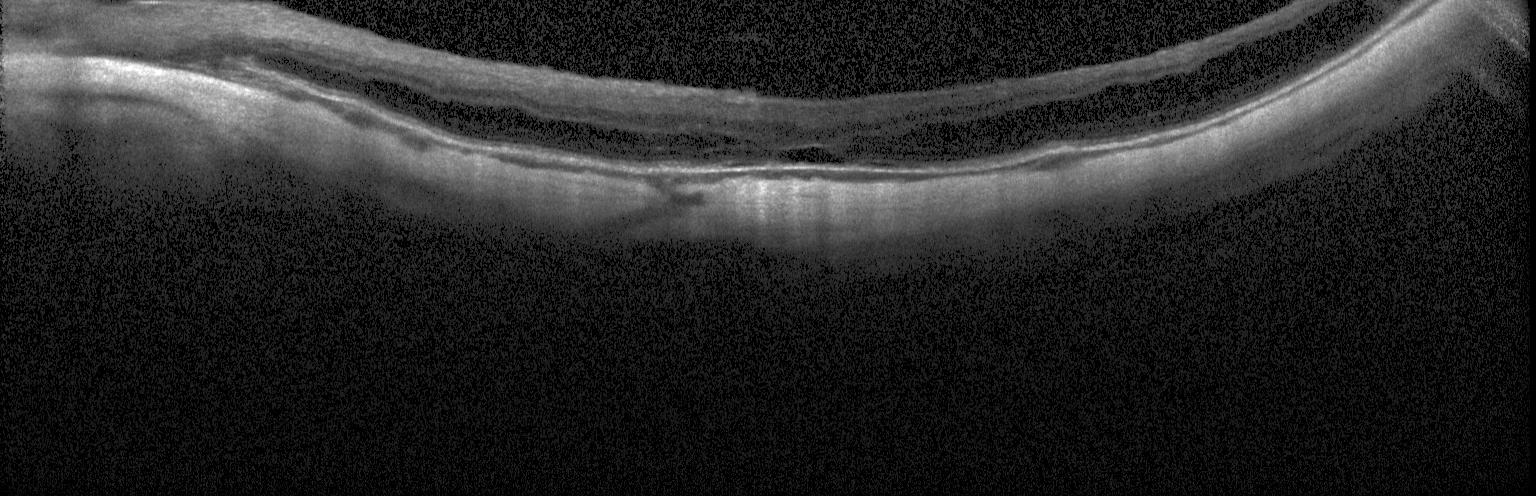 OCT B-scan.
Diagnosis: diabetic macular edema (DME).